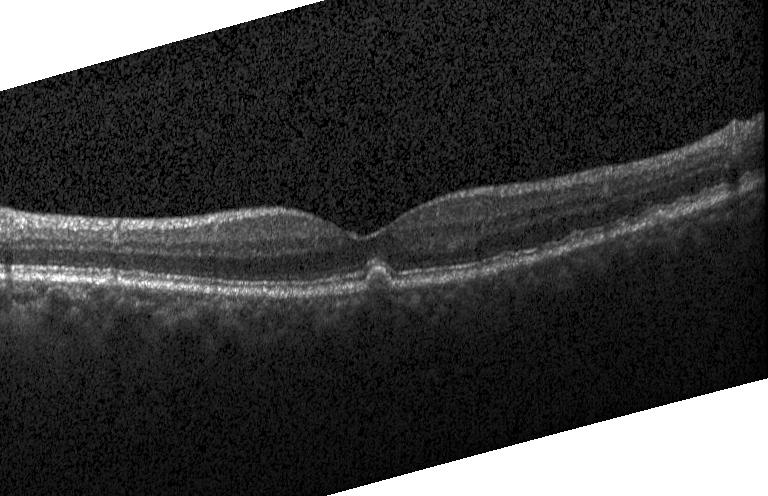

Optical coherence tomography scan · Heidelberg Spectralis. Drusen.